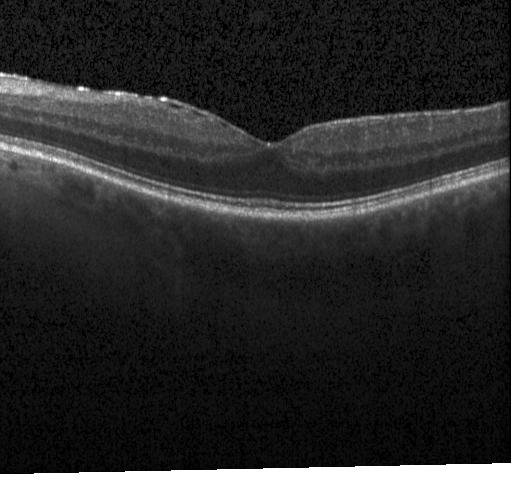 Optical coherence tomography scan — This B-scan demonstrates no evidence of CNV, DME, or drusen.